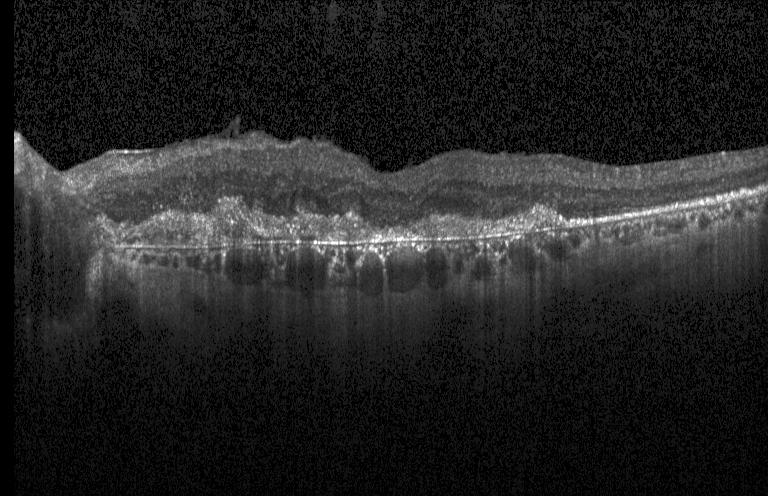
Optical coherence tomography B-scan, spectral-domain OCT, Heidelberg Spectralis, through the macula — OCT finding: choroidal neovascularization.